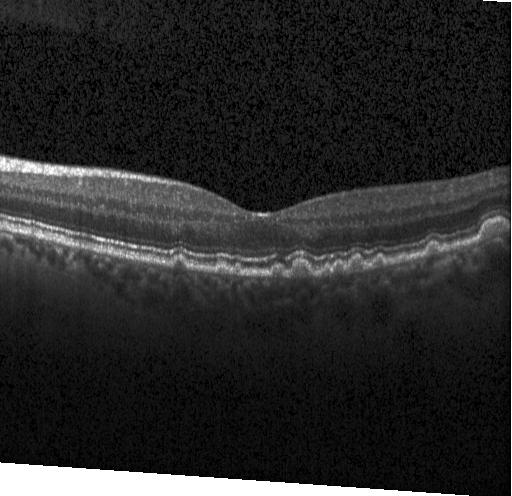

Dx: multiple drusen.